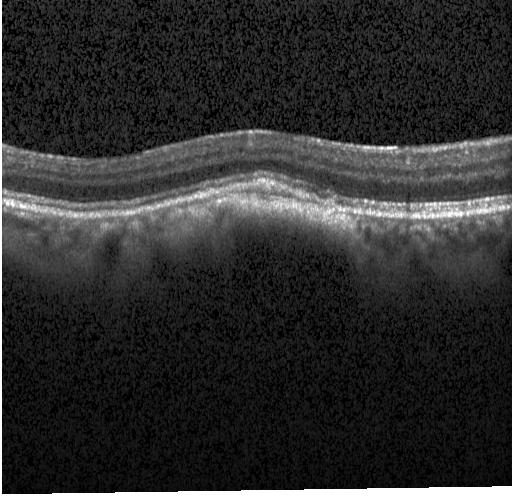 OCT line scan · horizontal scan through the fovea · spectral-domain OCT
Macular OCT: choroidal neovascularization.